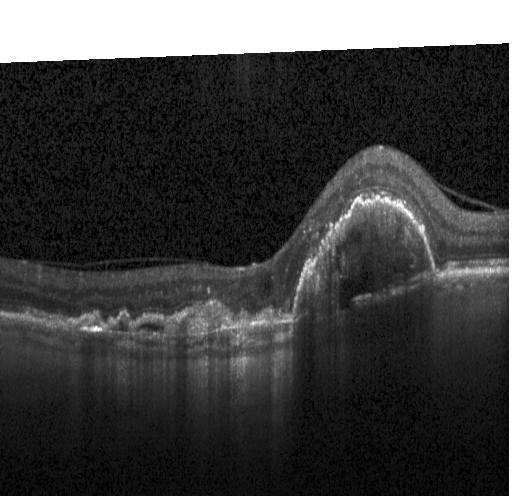 Retinal OCT B-scan. Acquired on a Heidelberg Spectralis — Diagnosis: choroidal neovascularization.